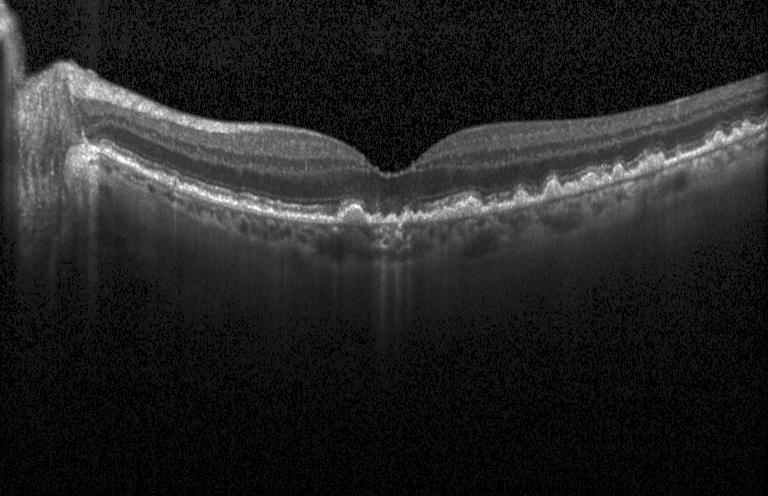
OCT finding: sub-RPE drusenoid deposits.